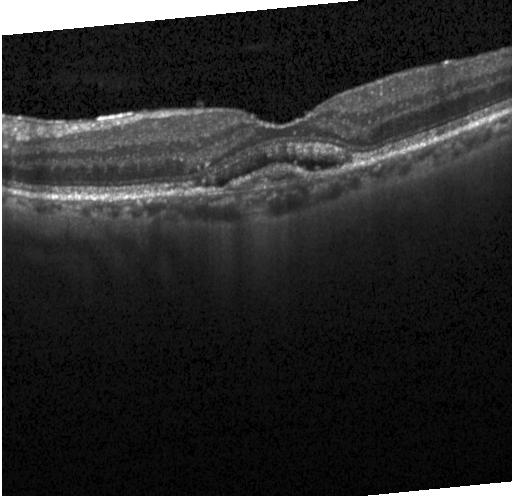

Retinal OCT B-scan; Heidelberg Spectralis. Macular OCT: CNV.